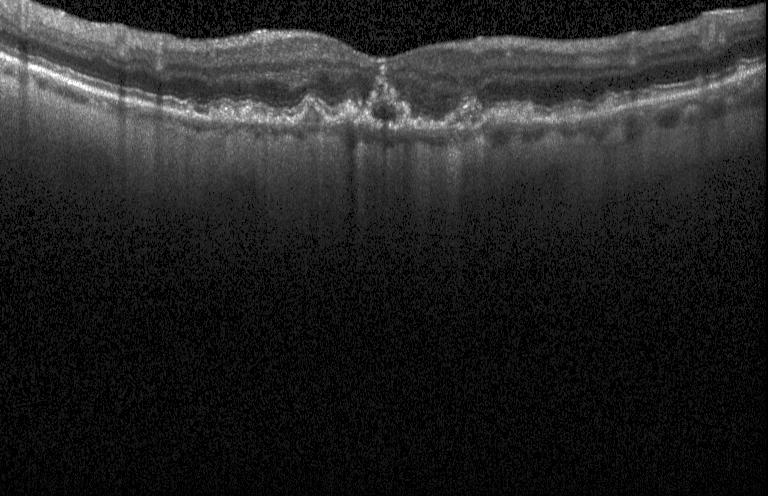

OCT B-scan, horizontal scan through the fovea, spectral-domain optical coherence tomography
The scan shows a choroidal neovascular membrane.